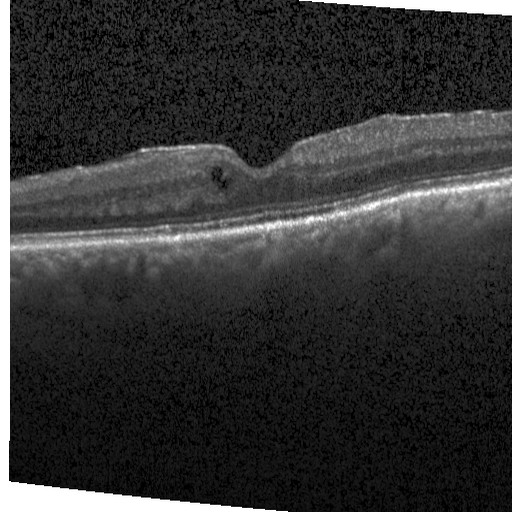 Heidelberg Spectralis OCT system; OCT line scan. Diagnosis: DME.